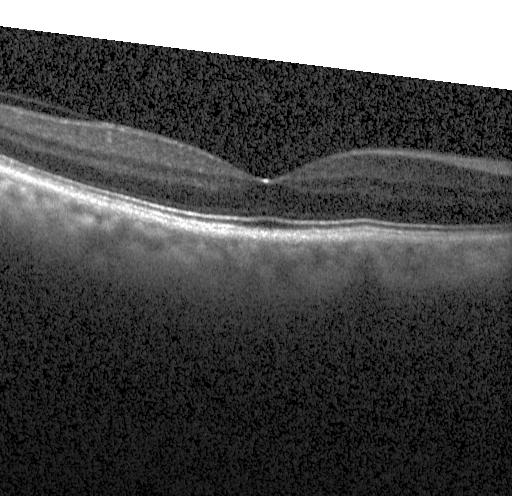
Retinal OCT cross-section showing no evidence of choroidal neovascularization, diabetic macular edema, or drusen.